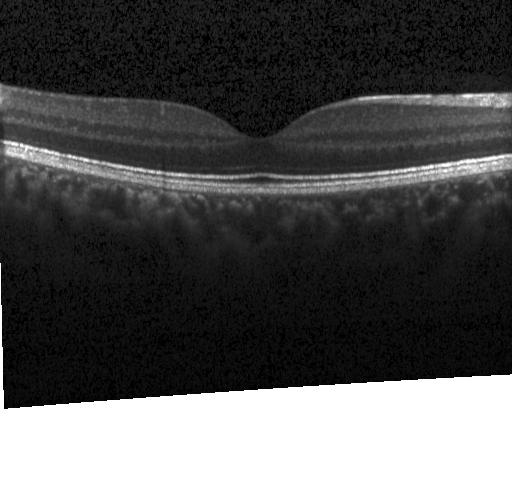
Optical coherence tomography scan · fovea-centered · instrument: Heidelberg Spectralis
Dx: neither choroidal neovascularization, diabetic macular edema, nor drusen.